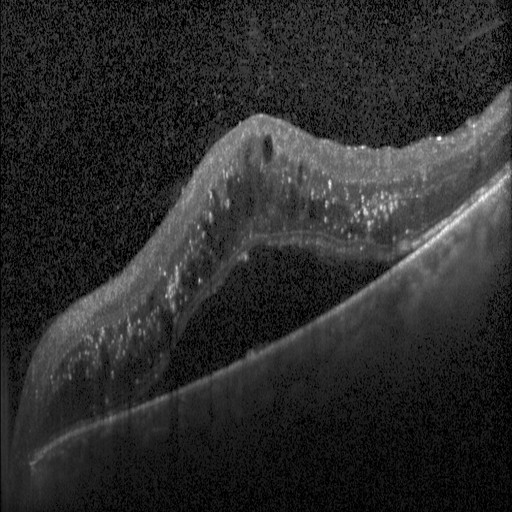 Macular OCT: DME.